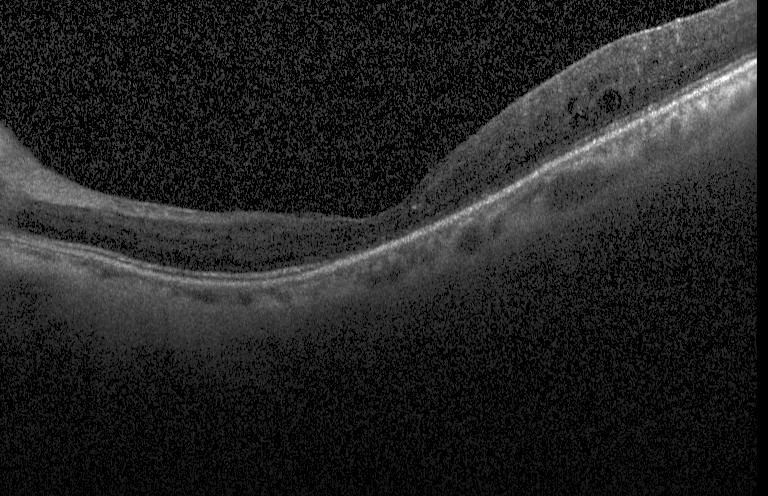
Retinal OCT B-scan, centered on the fovea. Finding: DME.